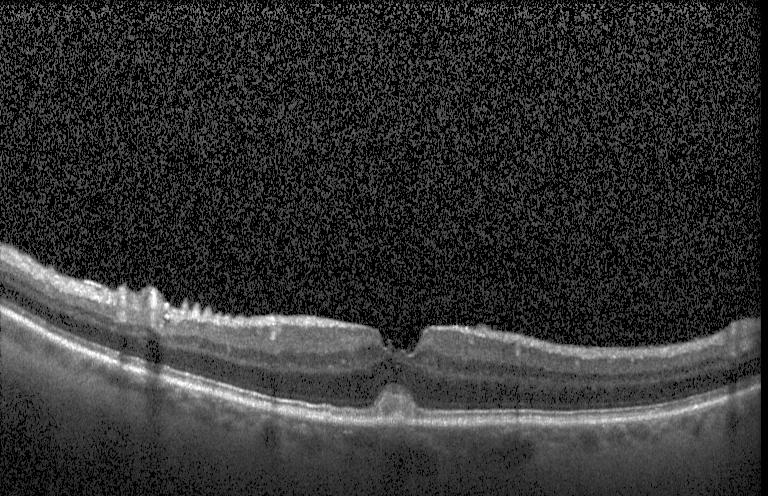 Impression: multiple drusen.